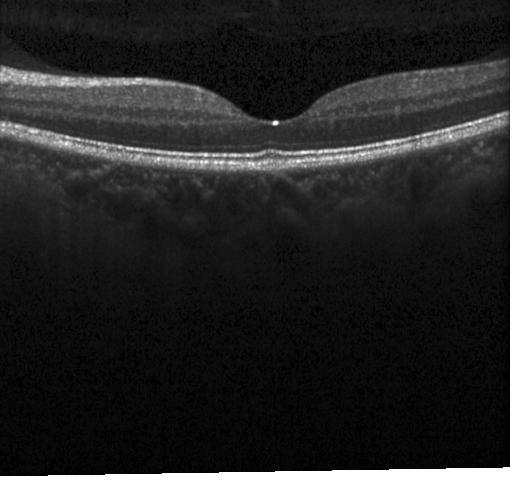
Instrument: Heidelberg Spectralis; macular scan; OCT line scan; SD-OCT
Dx: no choroidal neovascularization, no diabetic macular edema, and no drusen.